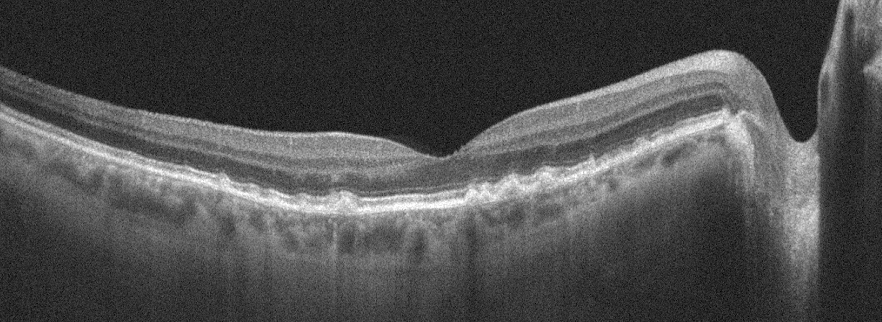
Retinal OCT cross-section, oculus dexter — Assessment: age-related macular degeneration (AMD).